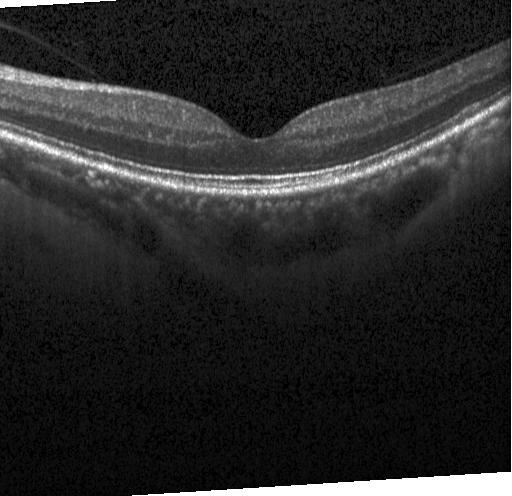
Retinal OCT cross-section. Finding: no CNV, DME, or drusen.